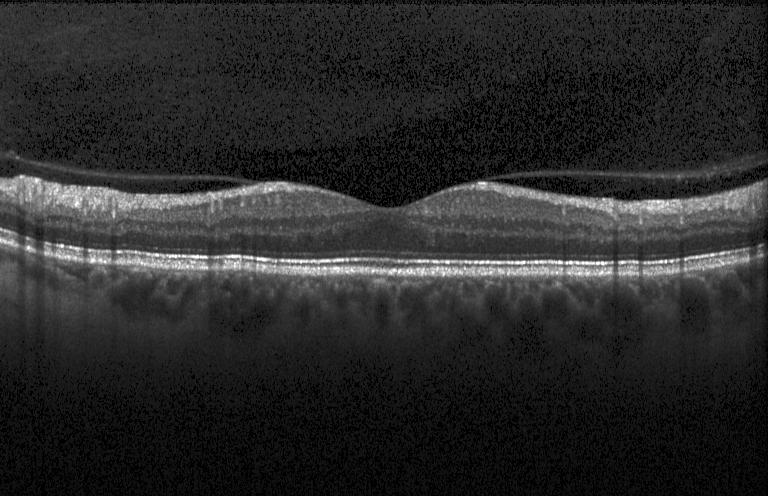
Optical coherence tomography scan · spectral-domain optical coherence tomography. Assessment: no choroidal neovascularization, no diabetic macular edema, and no drusen.